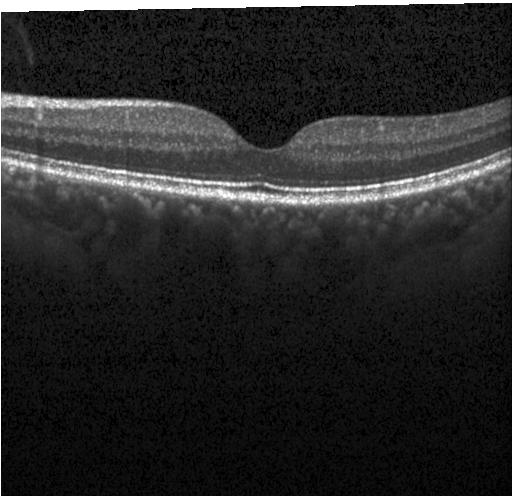
OCT line scan, Heidelberg Spectralis.
OCT finding: neither choroidal neovascularization, diabetic macular edema, nor drusen.